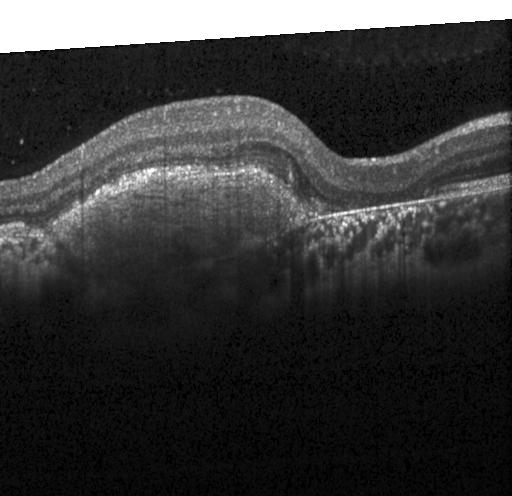 Centered on the fovea. OCT B-scan. Instrument: Heidelberg Spectralis — Impression: a choroidal neovascular membrane.